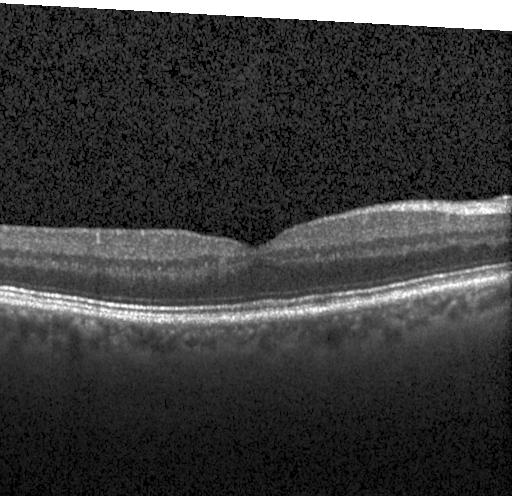 This B-scan demonstrates no evidence of choroidal neovascularization, diabetic macular edema, or drusen.